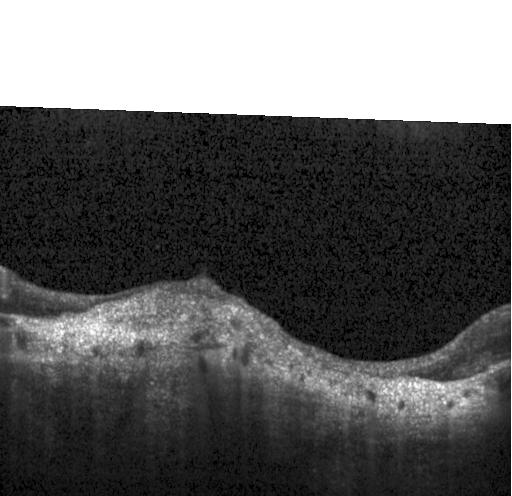

Horizontal scan through the fovea. Optical coherence tomography B-scan. Spectral-domain OCT — Finding: choroidal neovascularization (CNV).